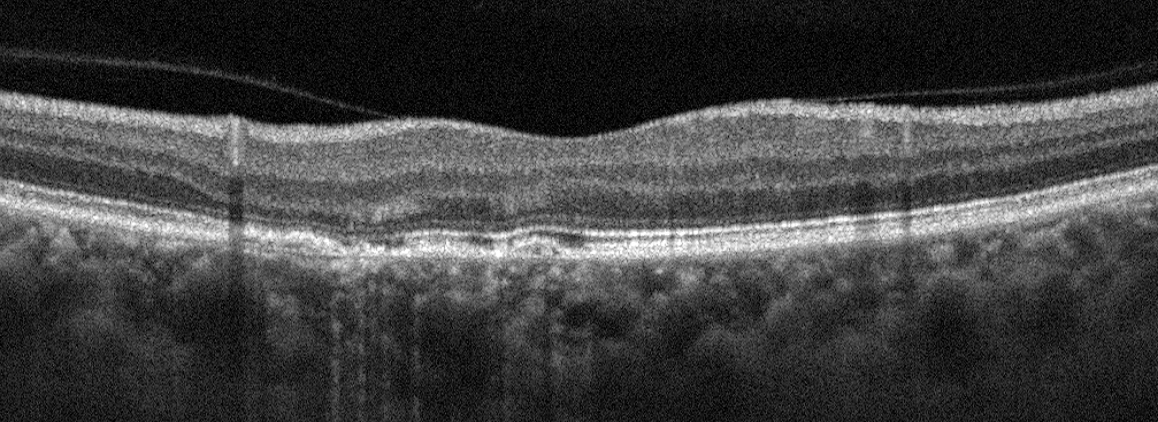
Left eye. Optical coherence tomography scan
Impression: age-related macular degeneration (AMD).